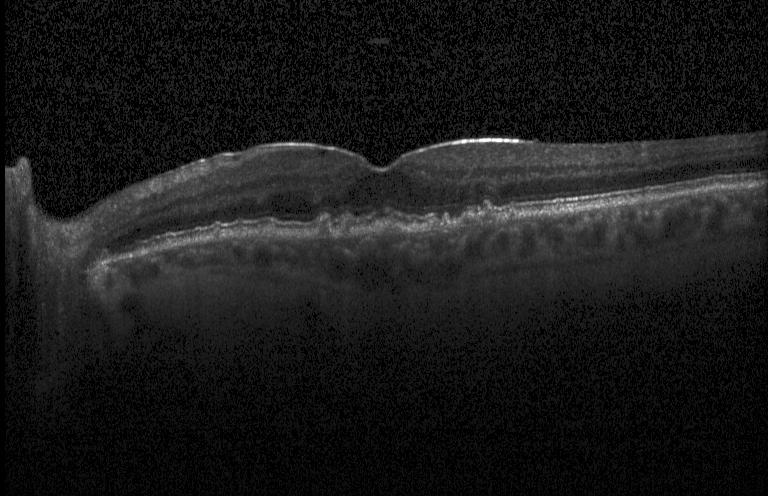
The scan shows drusen.